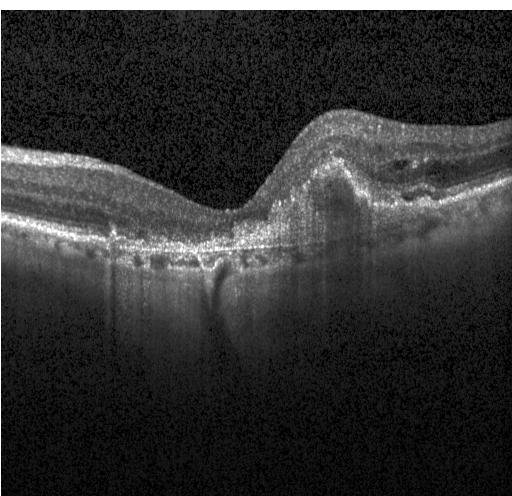
OCT B-scan. Spectral-domain OCT. Fovea-centered. A choroidal neovascular membrane.